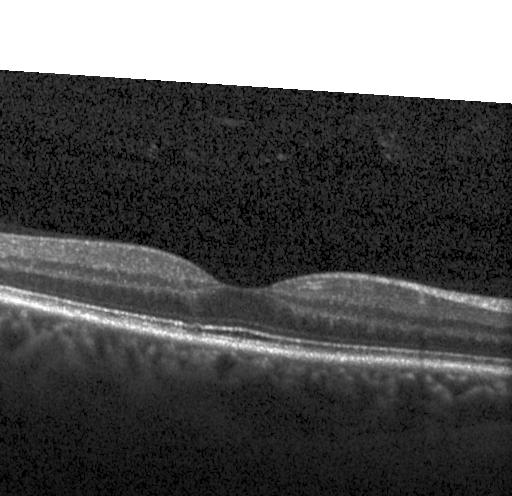
Centered on the fovea; spectral-domain optical coherence tomography; acquired on a Heidelberg Spectralis; retinal OCT cross-section — This B-scan demonstrates neither CNV, DME, nor drusen.